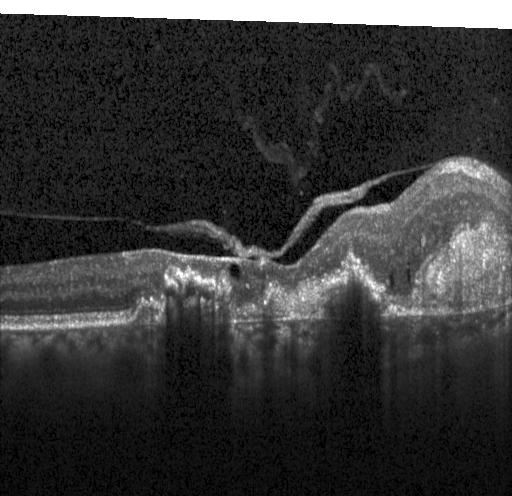

OCT B-scan · spectral-domain OCT
Finding: choroidal neovascularization (CNV).